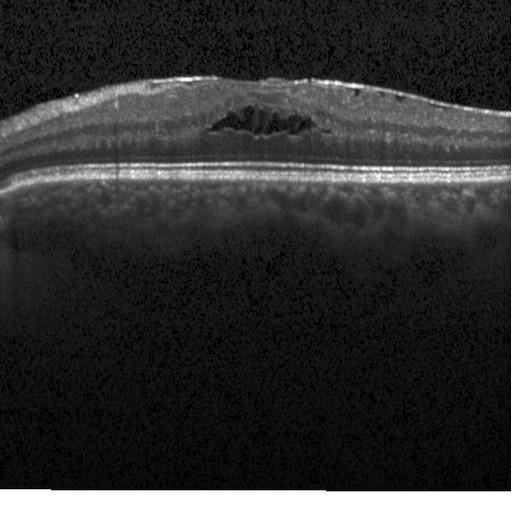 Retinal OCT B-scan — Finding: diabetic macular edema.